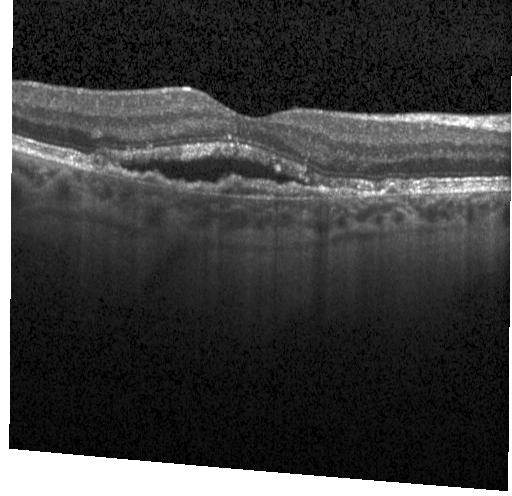

The scan shows a choroidal neovascular membrane.